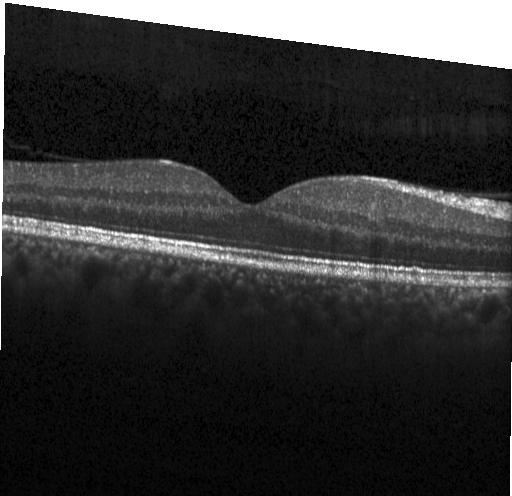 Horizontal scan through the fovea, instrument: Heidelberg Spectralis, optical coherence tomography scan, spectral-domain OCT
Diagnosis: no CNV, DME, or drusen.